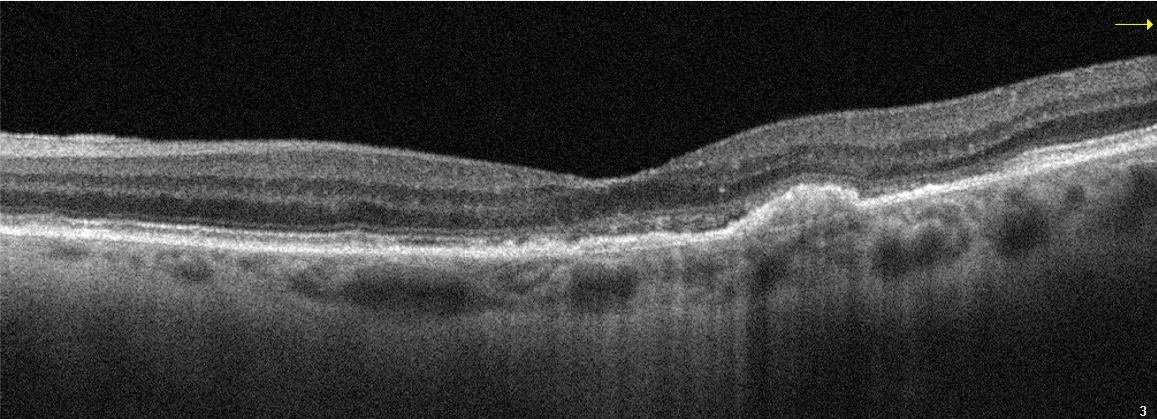

Optovue Avanti RTVue XR · optical coherence tomography B-scan · fovea-centered — Finding: AMD.